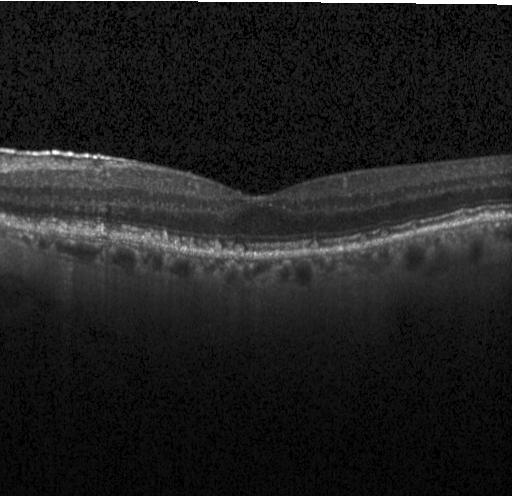

Through the macula; Heidelberg Spectralis; OCT line scan — Diagnosis: drusen.